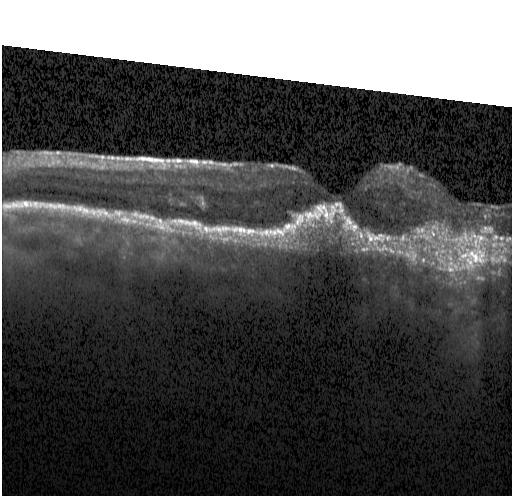 Choroidal neovascularization (CNV).